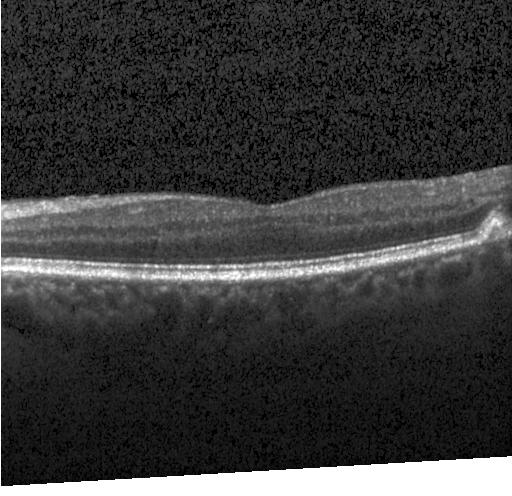

Retinal OCT B-scan. This B-scan demonstrates sub-RPE drusenoid deposits.